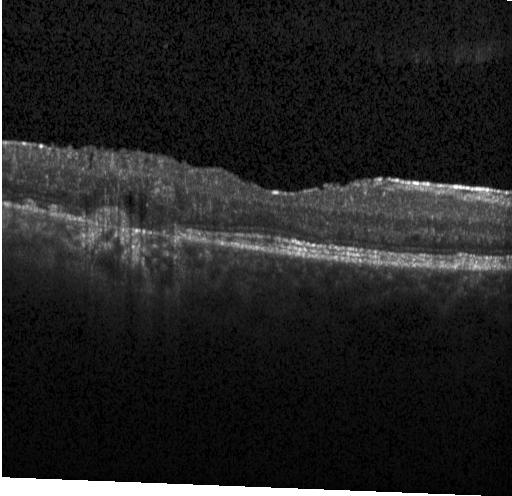 Retinal OCT cross-section — Finding: diabetic macular edema.